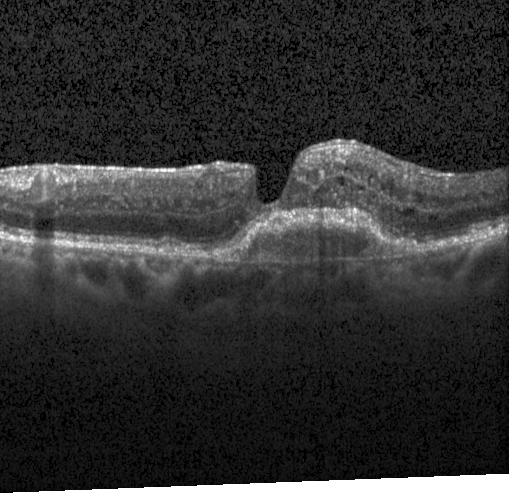

Optical coherence tomography scan — This B-scan demonstrates choroidal neovascularization.